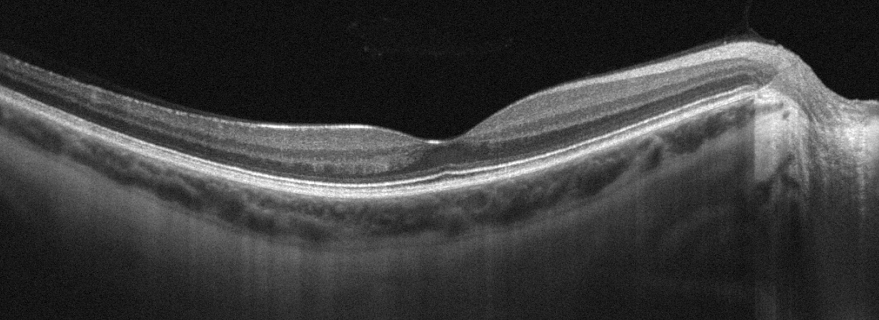

Diagnosis: no evidence of AMD, DME, ERM, RAO, RVO, or VID.